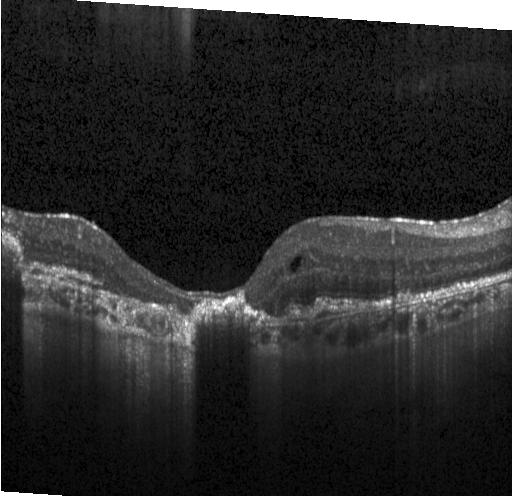
Through the macula · spectral-domain optical coherence tomography · OCT B-scan · instrument: Heidelberg Spectralis.
Dx: choroidal neovascularization (CNV).